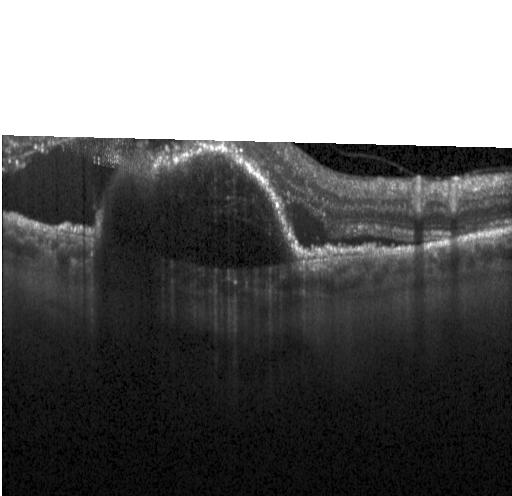

OCT B-scan. This B-scan demonstrates a choroidal neovascular membrane.